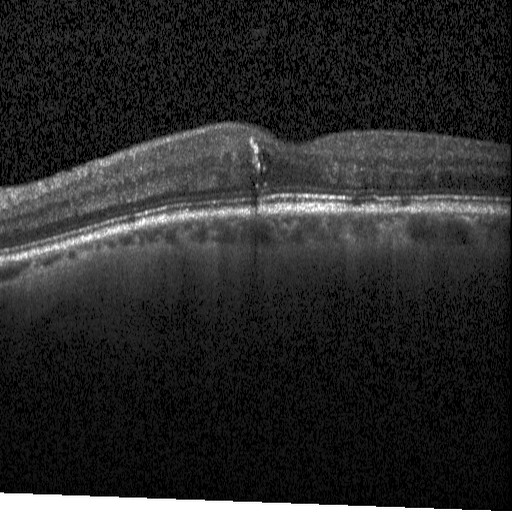 Macular OCT demonstrating diabetic macular edema (DME).